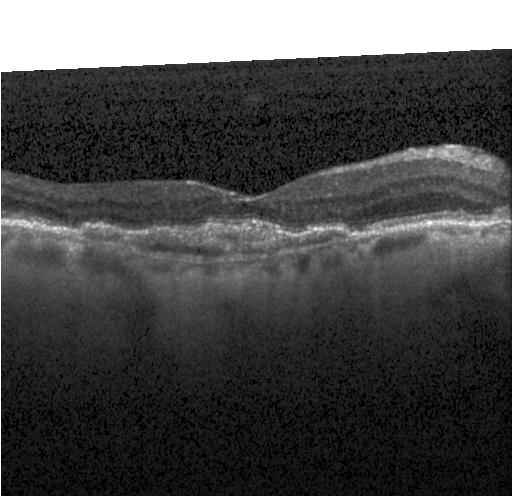 Acquired on a Heidelberg Spectralis; macular scan; SD-OCT; retinal OCT B-scan — Dx: a choroidal neovascular membrane.